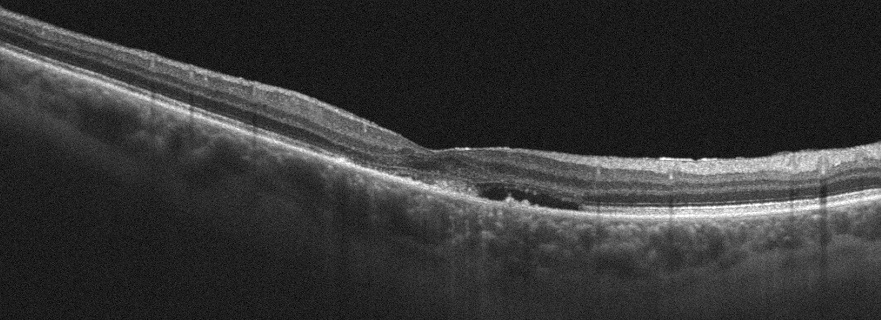 Through the macula, OCT B-scan, instrument: Optovue Avanti RTVue XR. Dx: AMD.